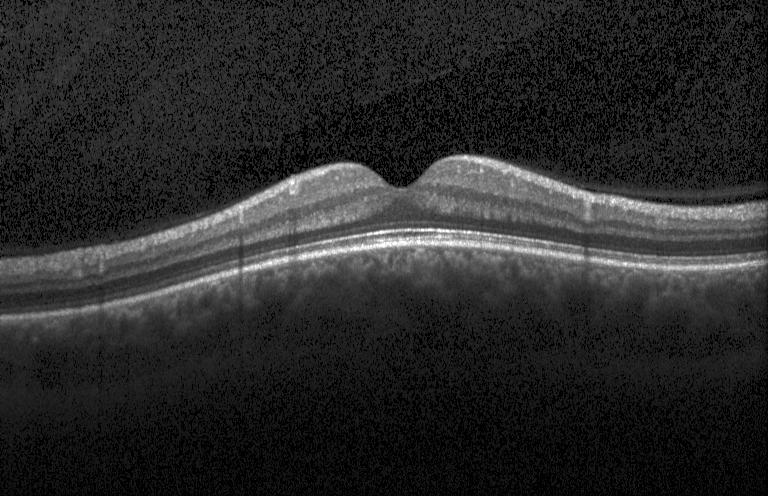
Retinal OCT B-scan.
This B-scan demonstrates no choroidal neovascularization, no diabetic macular edema, and no drusen.